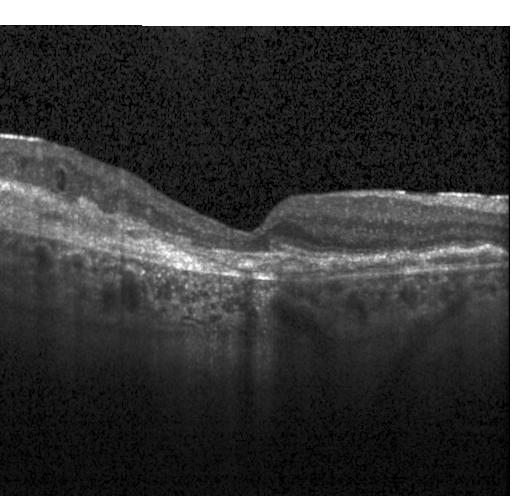 Macular OCT demonstrating a choroidal neovascular membrane.